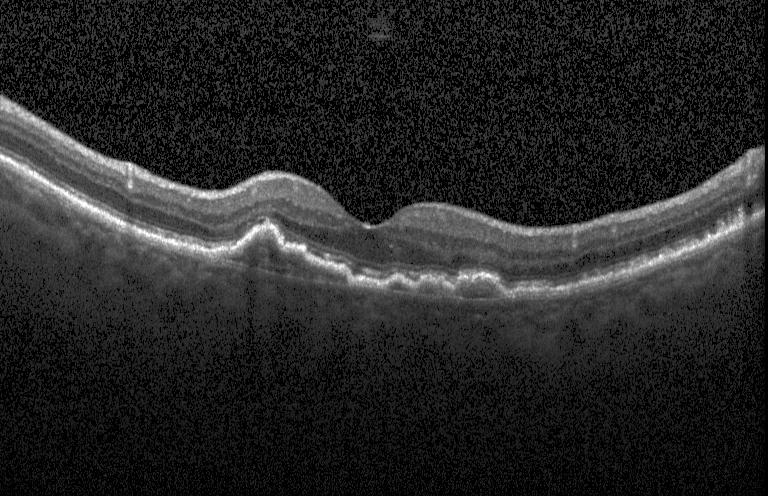
Optical coherence tomography scan · macular scan · Heidelberg Spectralis · spectral-domain optical coherence tomography. CNV.